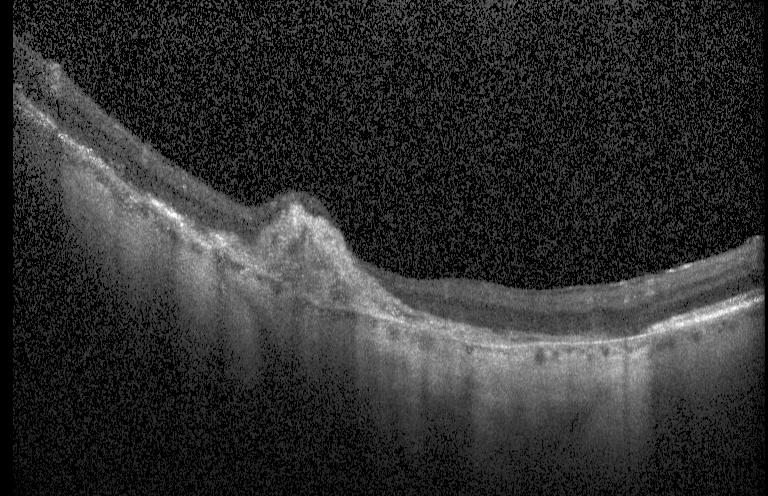

OCT B-scan showing a choroidal neovascular membrane.